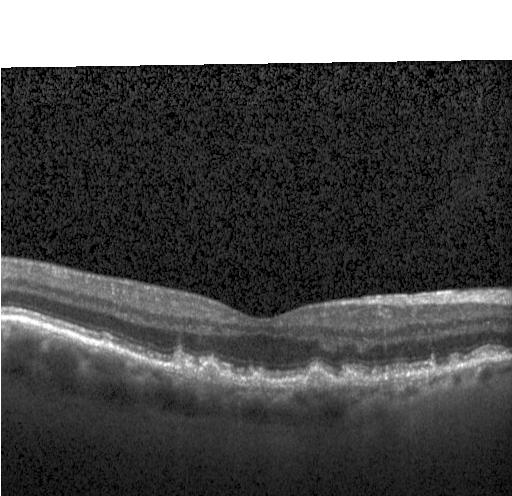
Macular scan. Optical coherence tomography B-scan. Spectral-domain optical coherence tomography. Assessment: multiple drusen.